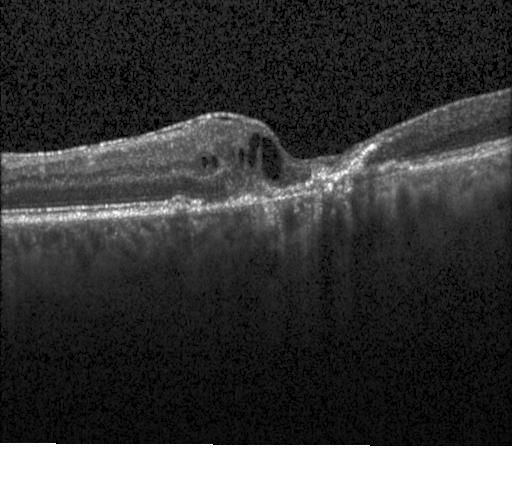

Spectral-domain OCT · acquired on a Heidelberg Spectralis · OCT line scan · macular scan
Diagnosis: choroidal neovascularization (CNV).